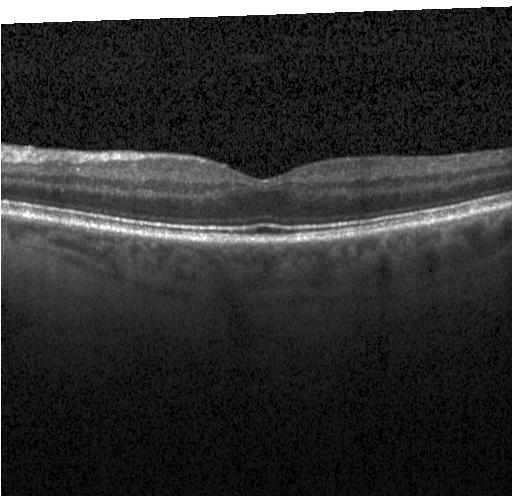

OCT line scan.
The scan shows no evidence of CNV, DME, or drusen.